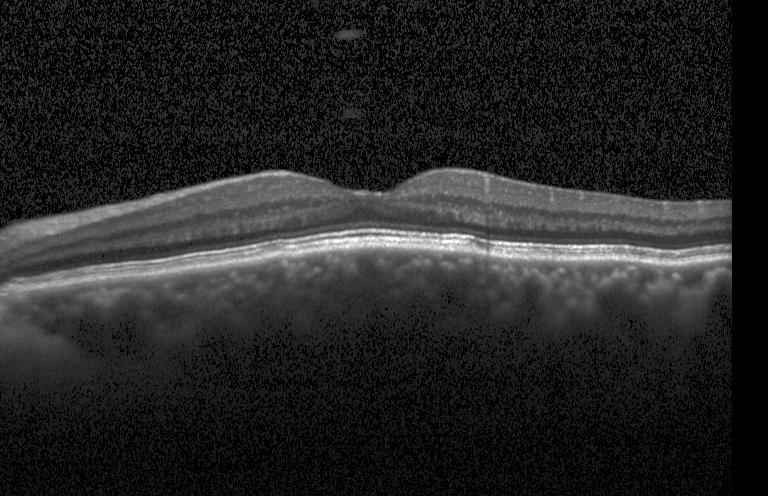 OCT scan showing no evidence of choroidal neovascularization, diabetic macular edema, or drusen.